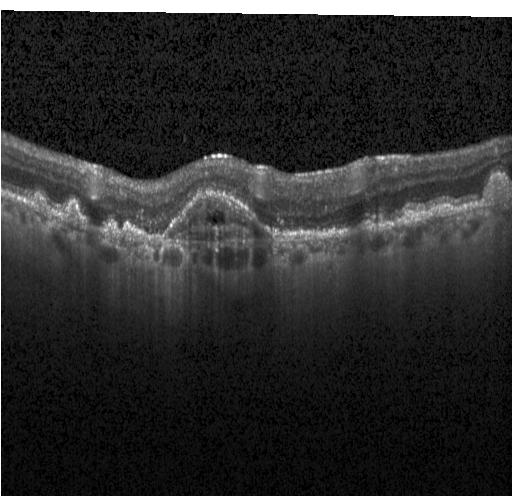 Instrument: Heidelberg Spectralis; retinal OCT cross-section; SD-OCT; through the macula. The scan shows choroidal neovascularization (CNV).